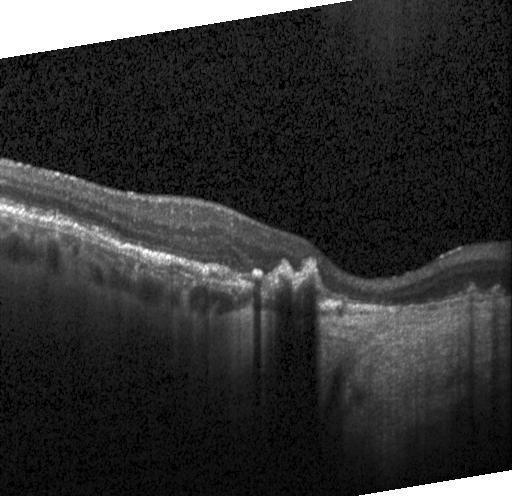 Heidelberg Spectralis, OCT B-scan, centered on the fovea — Diagnosis: a choroidal neovascular membrane.